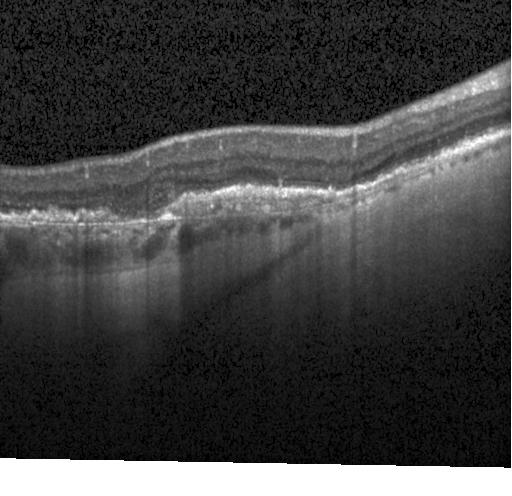
OCT B-scan, SD-OCT, instrument: Heidelberg Spectralis, through the macula. OCT finding: a choroidal neovascular membrane.